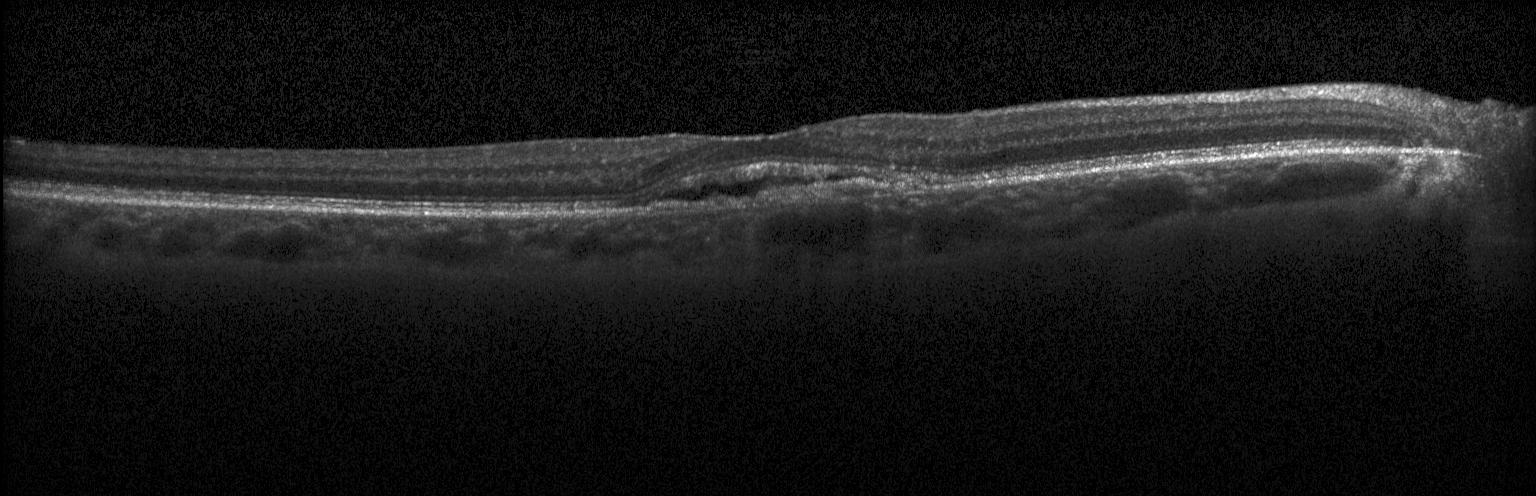 This B-scan demonstrates CNV.